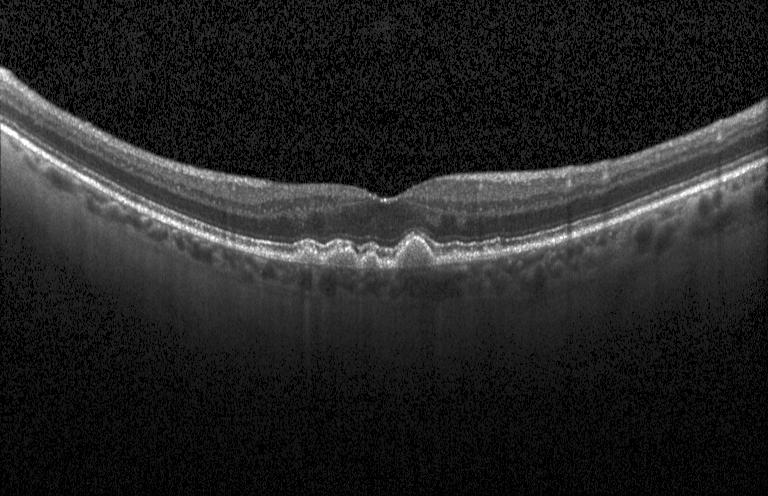 Diagnosis: drusen.